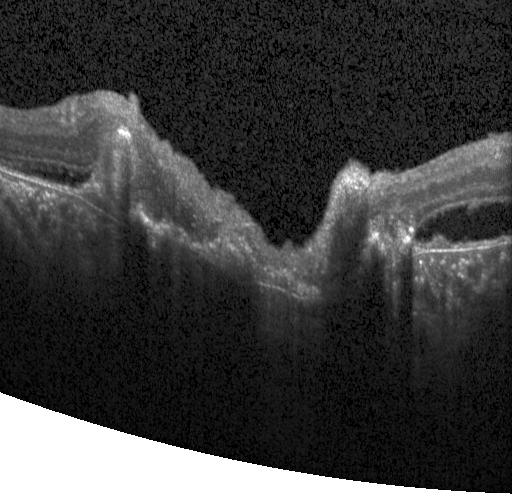 SD-OCT. Retinal OCT cross-section
Macular OCT: a choroidal neovascular membrane.